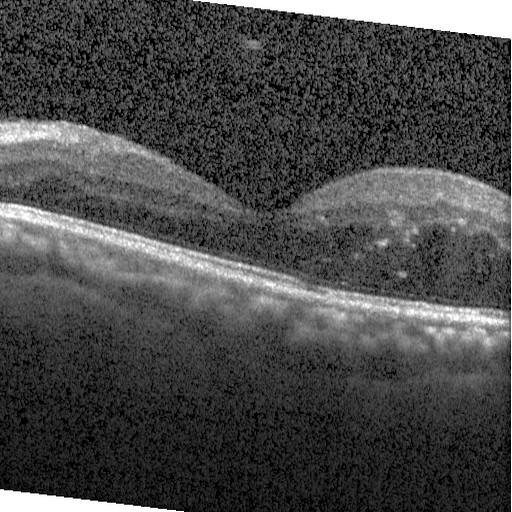 Macular scan · retinal OCT cross-section · Heidelberg Spectralis — Macular OCT: diabetic macular edema (DME).